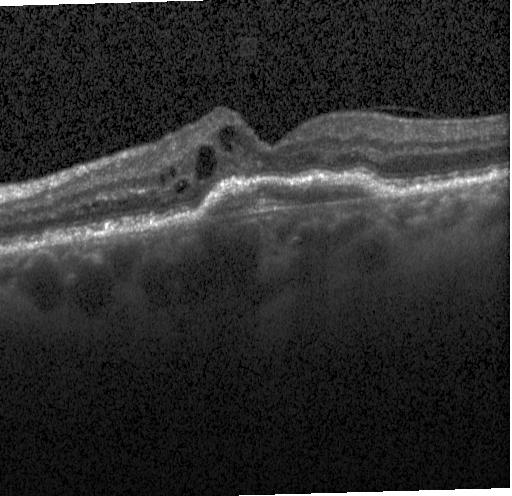 Spectral-domain OCT; OCT B-scan.
This B-scan demonstrates a choroidal neovascular membrane.